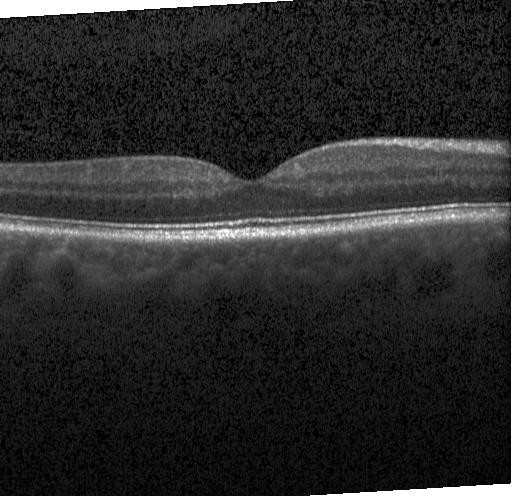

Impression: no evidence of CNV, DME, or drusen.